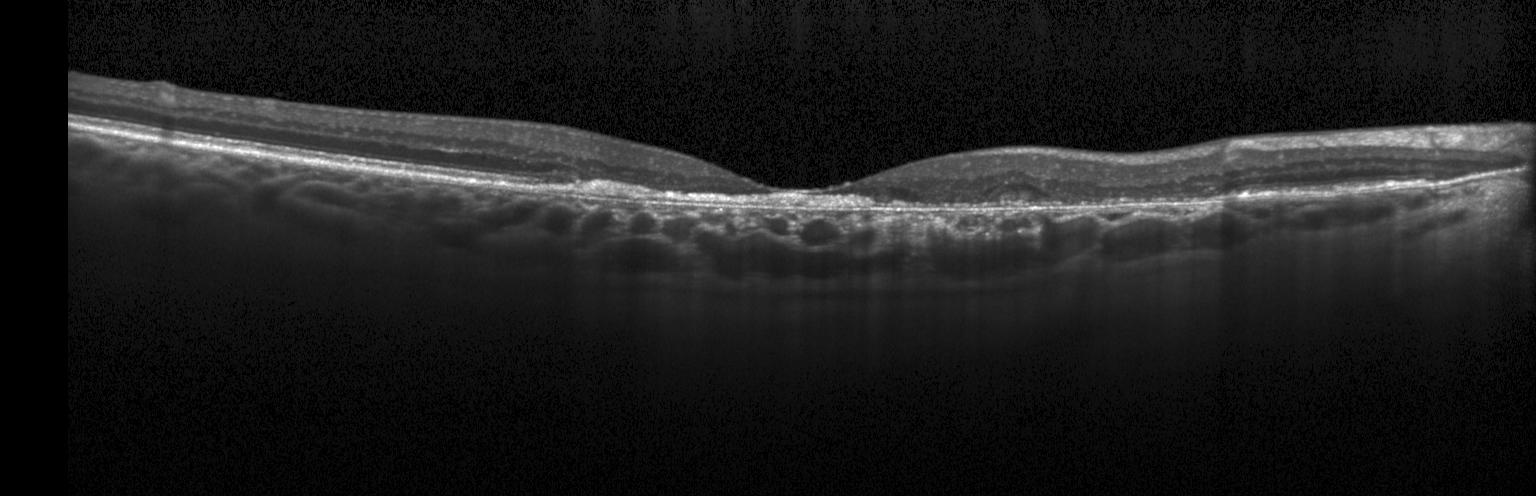

Assessment: choroidal neovascularization.